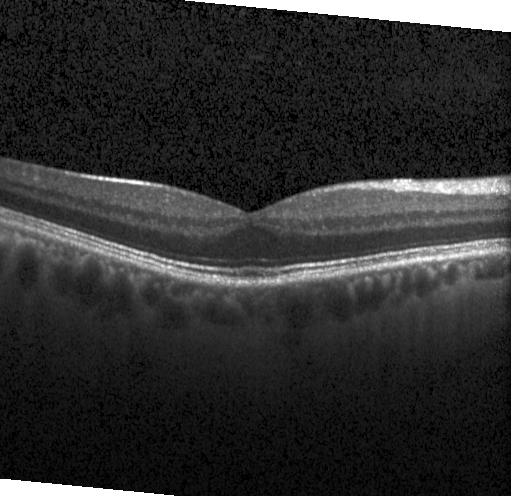 Fovea-centered · retinal OCT cross-section — OCT finding: no choroidal neovascularization, diabetic macular edema, or drusen.